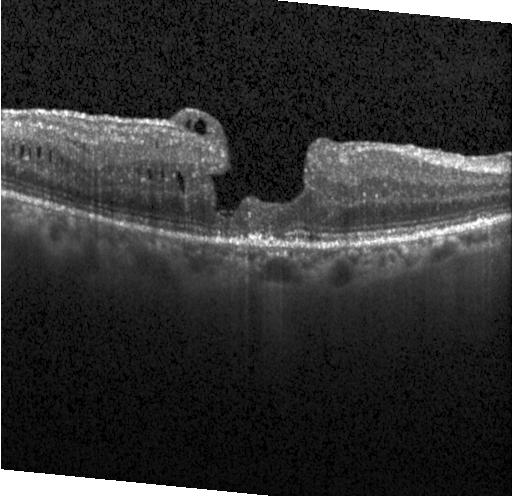

Finding: diabetic macular edema.